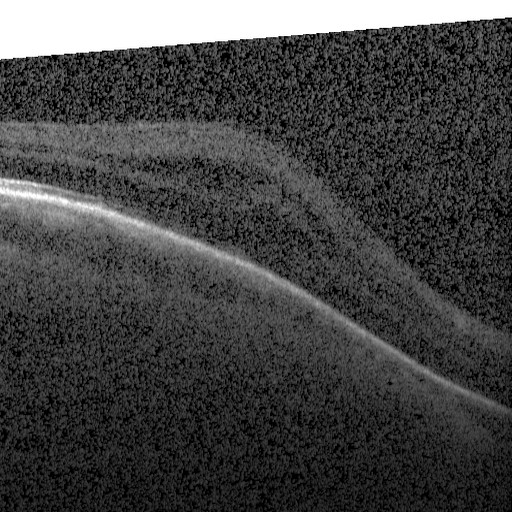

Retinal OCT cross-section showing diabetic macular edema (DME).